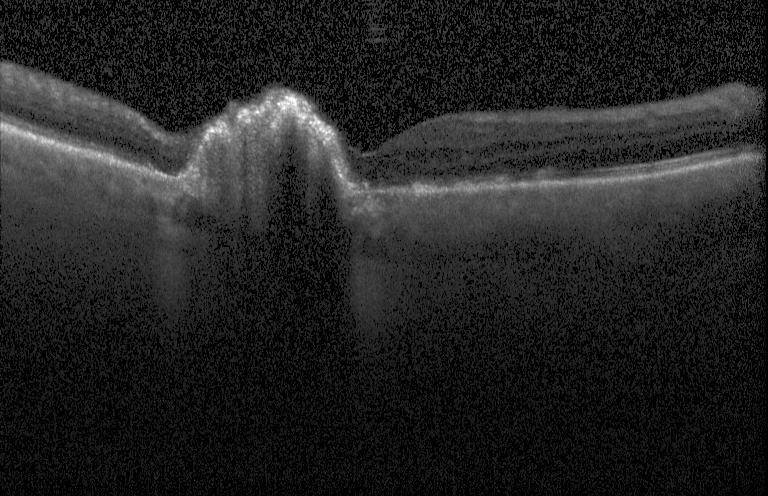

This B-scan demonstrates a choroidal neovascular membrane.